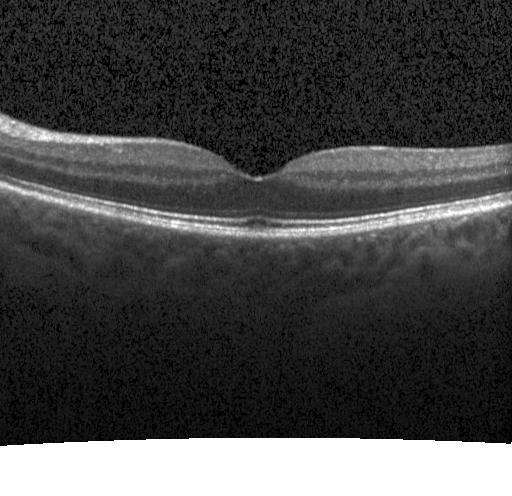 Centered on the fovea · Heidelberg Spectralis · OCT B-scan
OCT finding: neither CNV, DME, nor drusen.